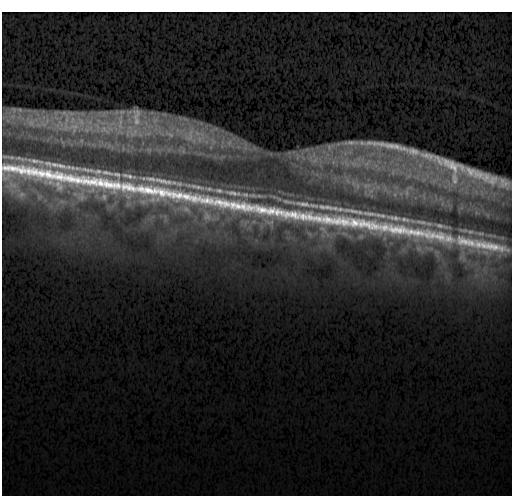 Retinal OCT B-scan, acquired on a Heidelberg Spectralis
Diagnosis: neither choroidal neovascularization, diabetic macular edema, nor drusen.